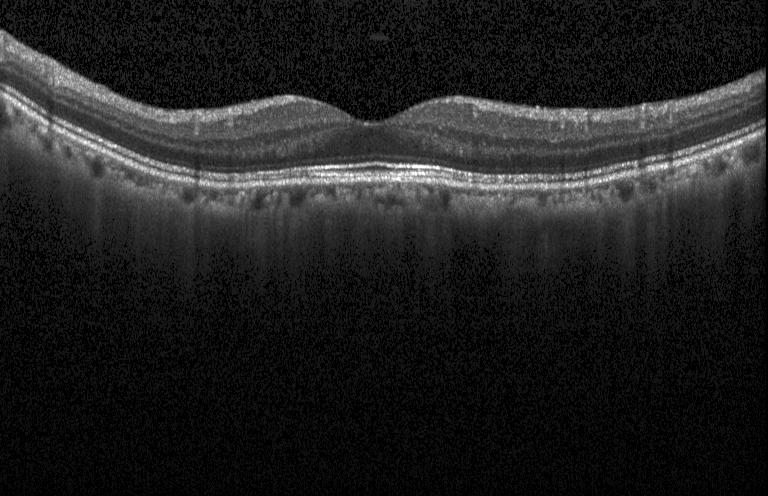
Macular scan · retinal OCT B-scan · SD-OCT · Heidelberg Spectralis. Diagnosis: neither CNV, DME, nor drusen.